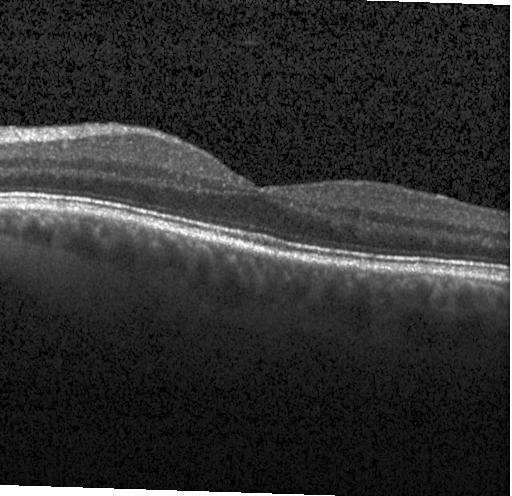 Fovea-centered, Heidelberg Spectralis, OCT B-scan, spectral-domain OCT.
The scan shows neither CNV, DME, nor drusen.